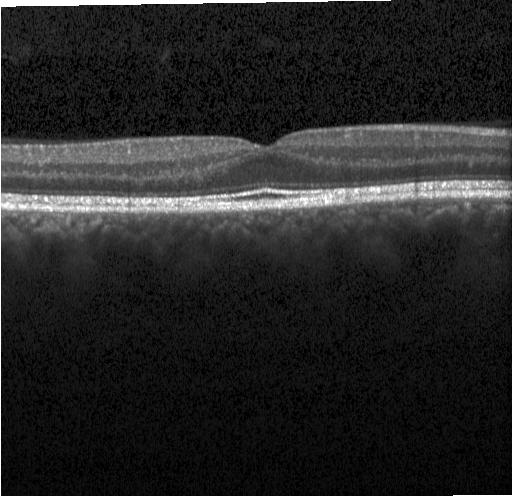

Assessment: no evidence of choroidal neovascularization, diabetic macular edema, or drusen.